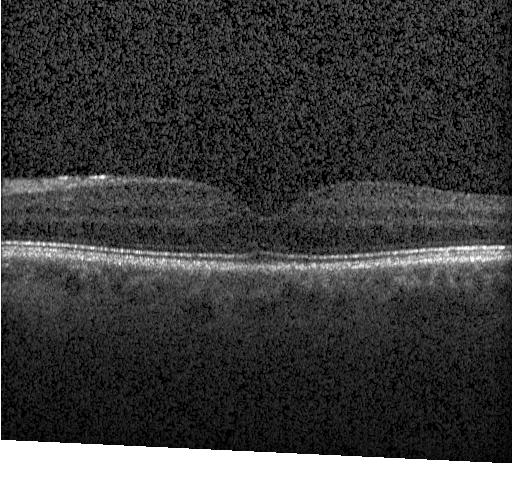 Retinal OCT cross-section; SD-OCT; fovea-centered; Heidelberg Spectralis OCT system — Finding: no CNV, DME, or drusen.